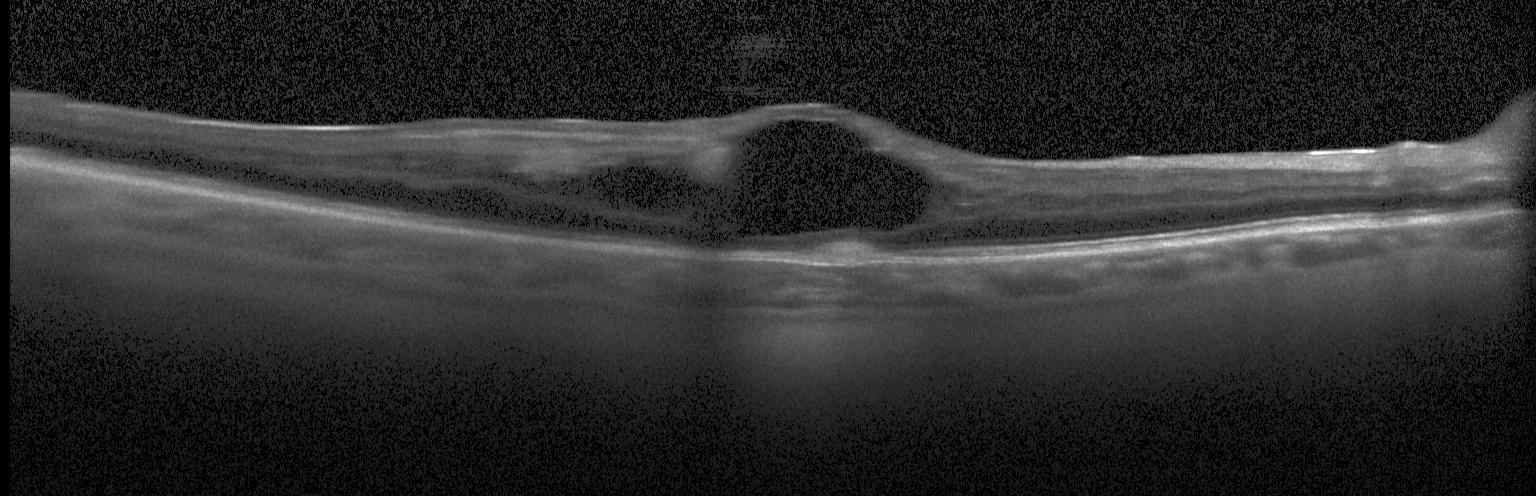
Retinal OCT cross-section showing CNV.